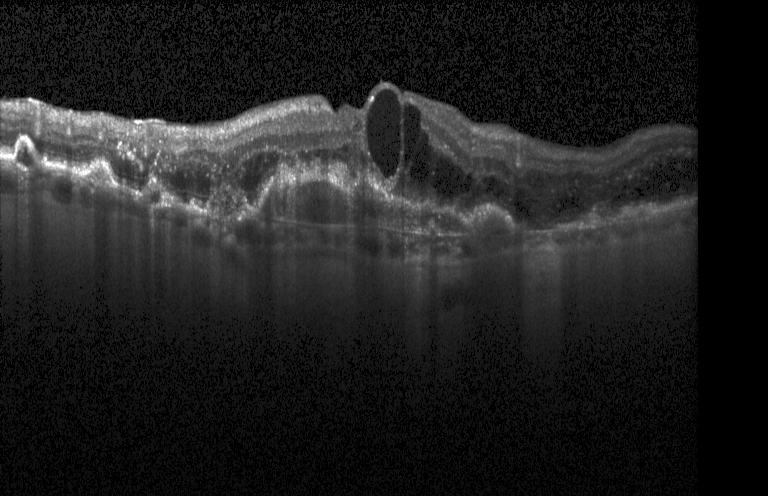

Spectral-domain optical coherence tomography. Optical coherence tomography scan
Impression: choroidal neovascularization.